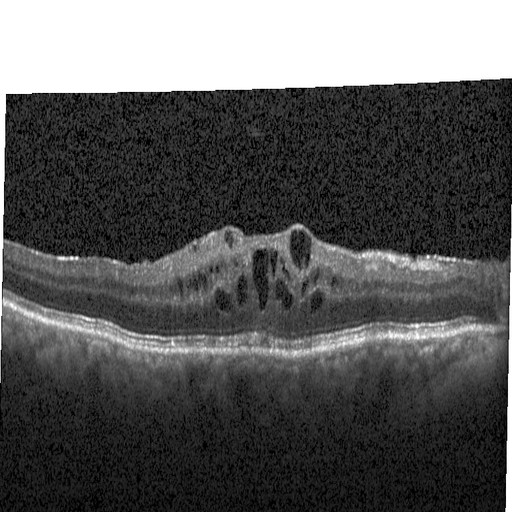
Macular OCT: diabetic macular edema.